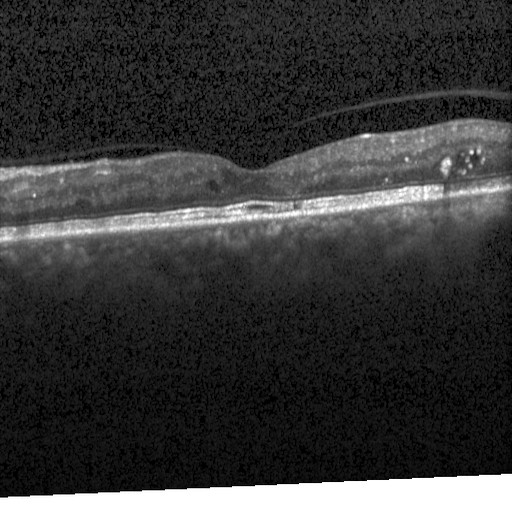
OCT B-scan — DME.